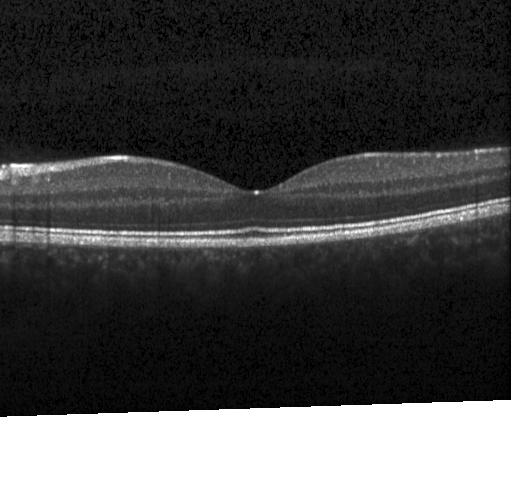

Horizontal scan through the fovea · spectral-domain OCT · optical coherence tomography B-scan · acquired on a Heidelberg Spectralis.
Neither choroidal neovascularization, diabetic macular edema, nor drusen.